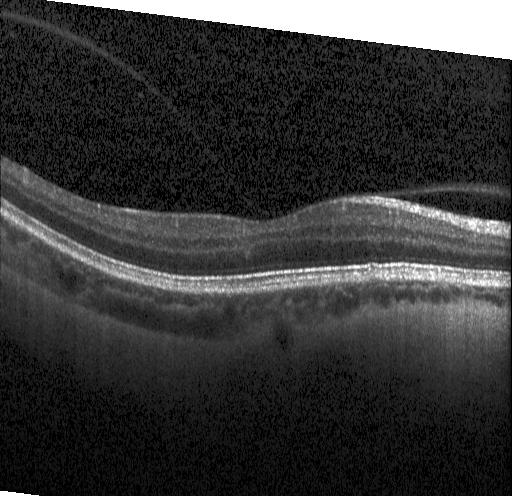
OCT finding: no choroidal neovascularization, no diabetic macular edema, and no drusen.